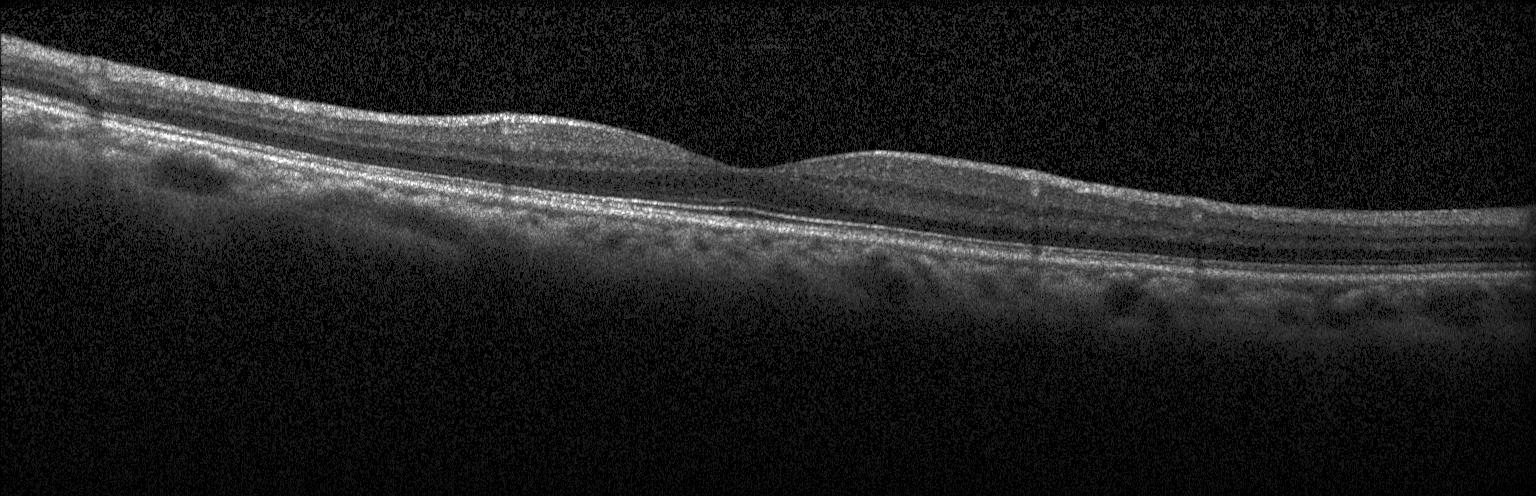
Optical coherence tomography B-scan — Finding: no CNV, no DME, and no drusen.